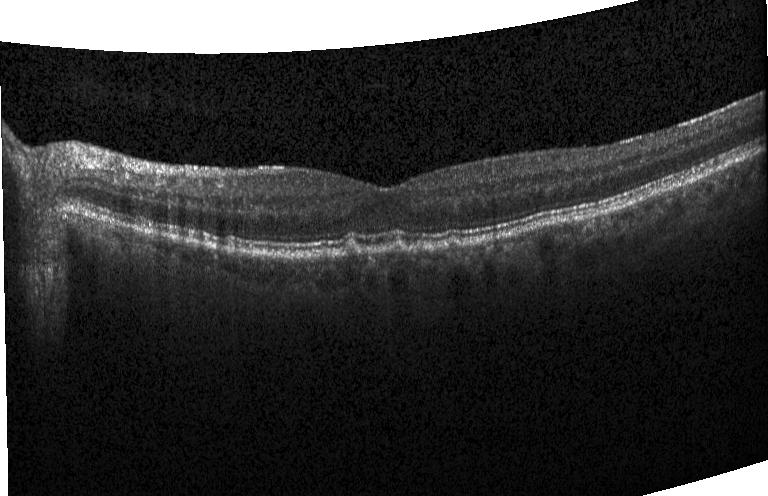 Fovea-centered. OCT line scan. Instrument: Heidelberg Spectralis. OCT finding: sub-RPE drusenoid deposits.